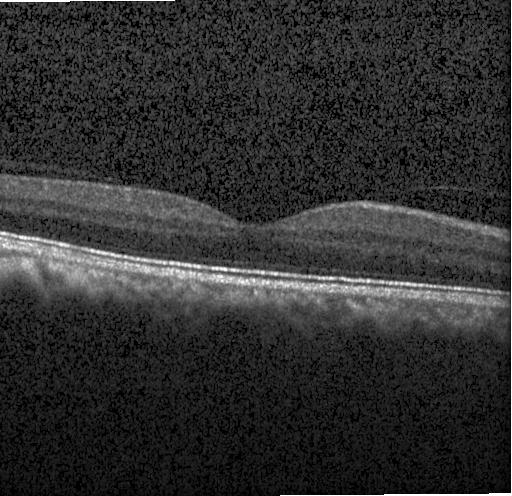

Horizontal scan through the fovea · acquired on a Heidelberg Spectralis · retinal OCT B-scan.
Impression: neither CNV, DME, nor drusen.